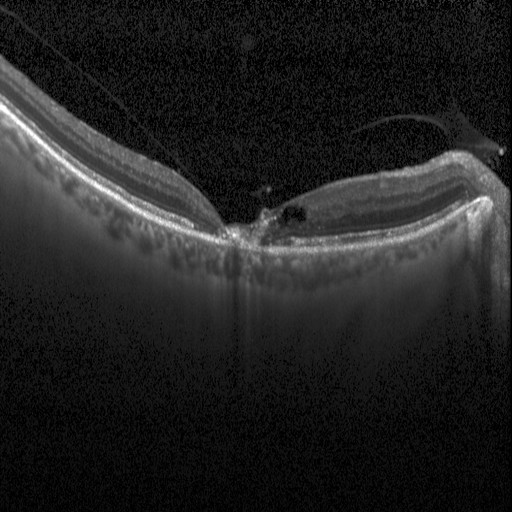 Spectral-domain optical coherence tomography · Heidelberg Spectralis · retinal OCT B-scan.
The scan shows DME.